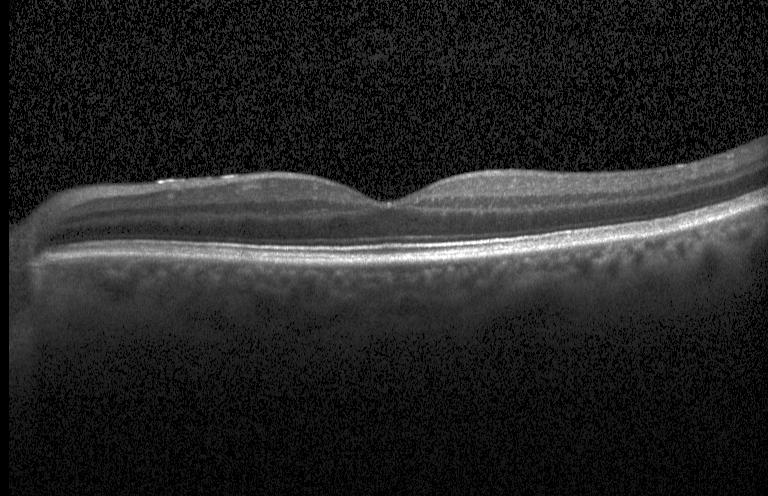 Heidelberg Spectralis. OCT line scan — Assessment: no CNV, no DME, and no drusen.